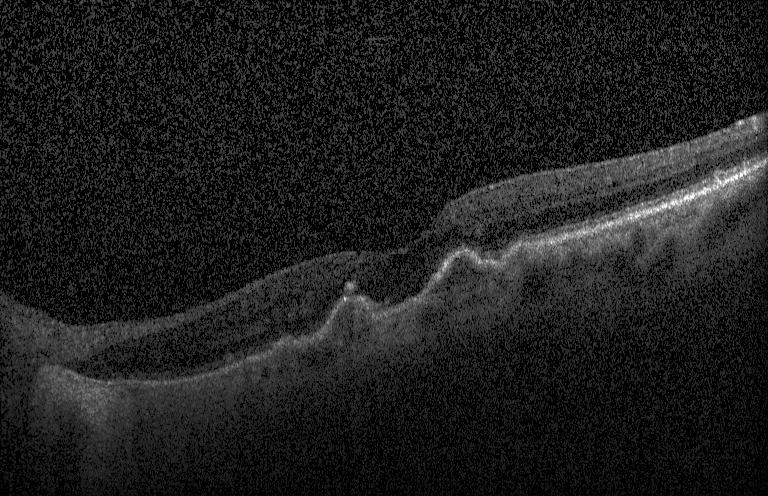 Optical coherence tomography scan. This B-scan demonstrates choroidal neovascularization.